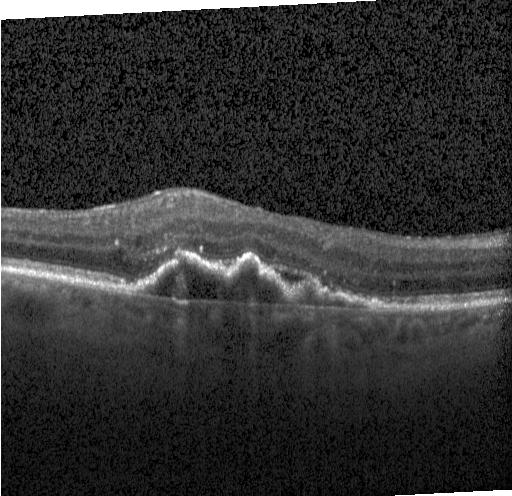 Macular OCT: a choroidal neovascular membrane.